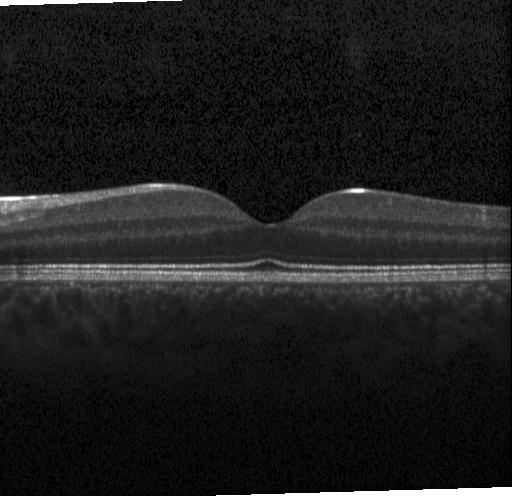 No evidence of CNV, DME, or drusen.